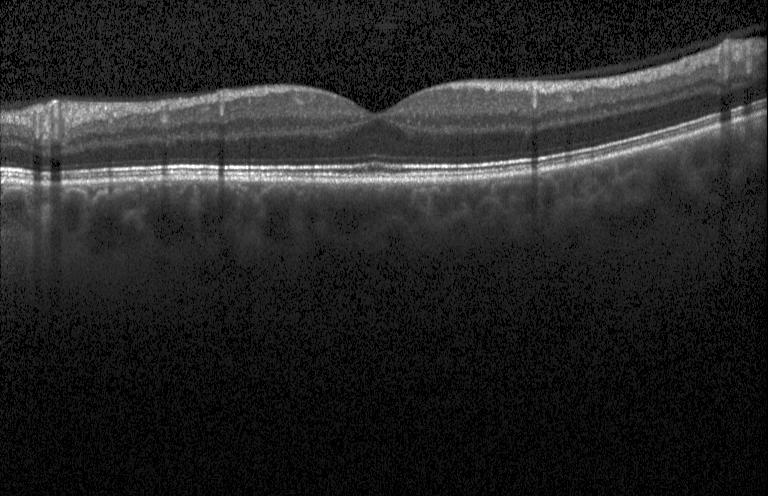
Retinal OCT cross-section, acquired on a Heidelberg Spectralis — Diagnosis: no evidence of CNV, DME, or drusen.